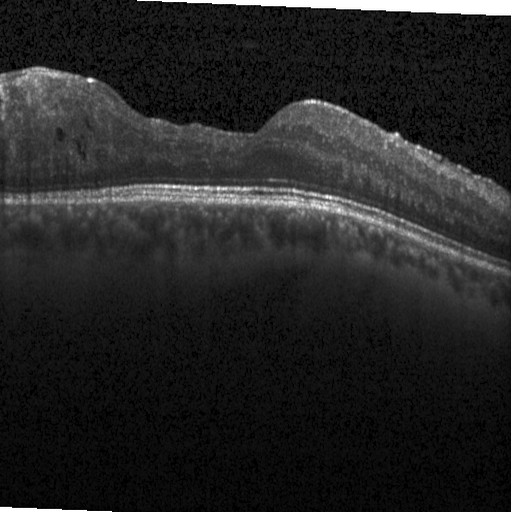

Assessment: diabetic macular edema.